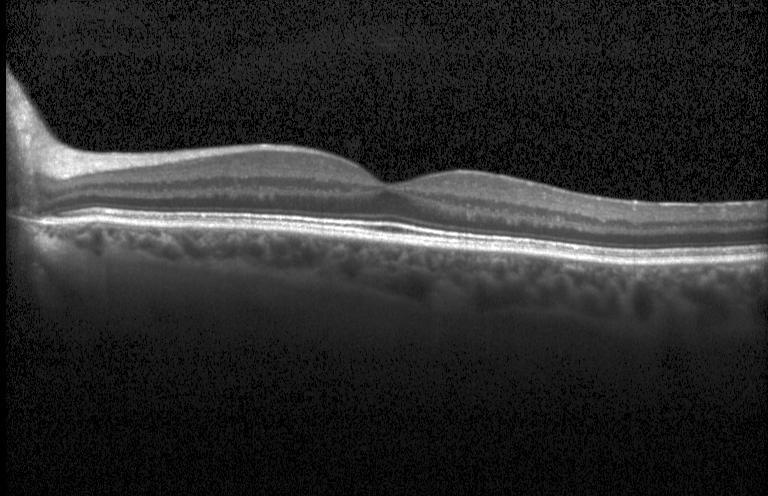
Impression: no evidence of choroidal neovascularization, diabetic macular edema, or drusen.